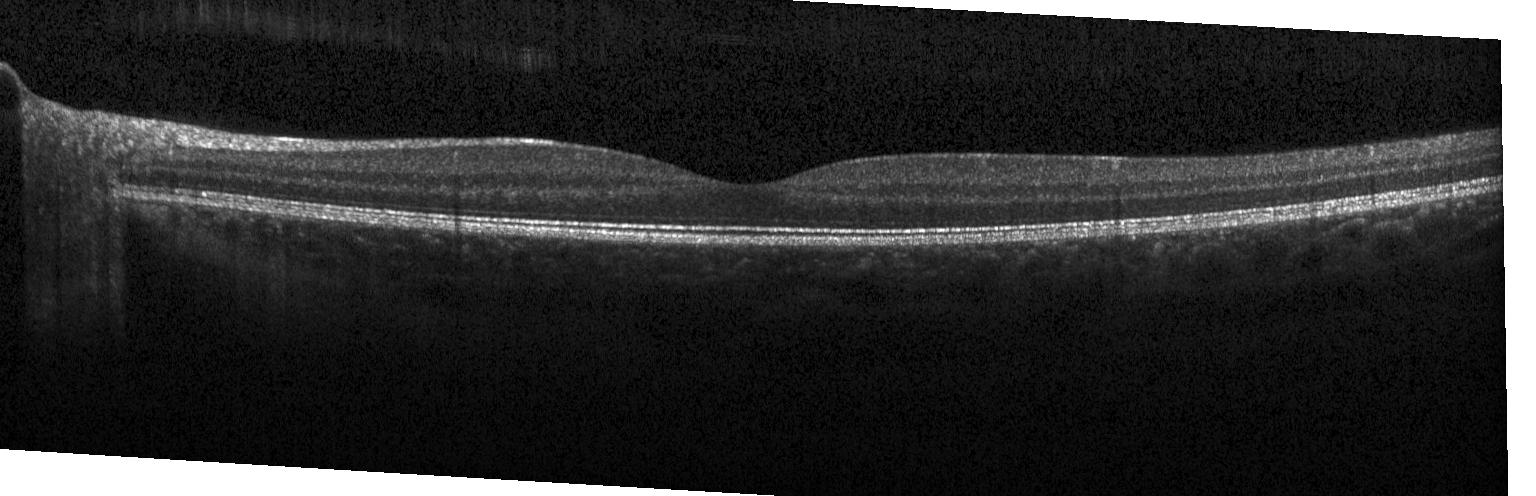 Fovea-centered, retinal OCT B-scan.
Dx: no evidence of CNV, DME, or drusen.